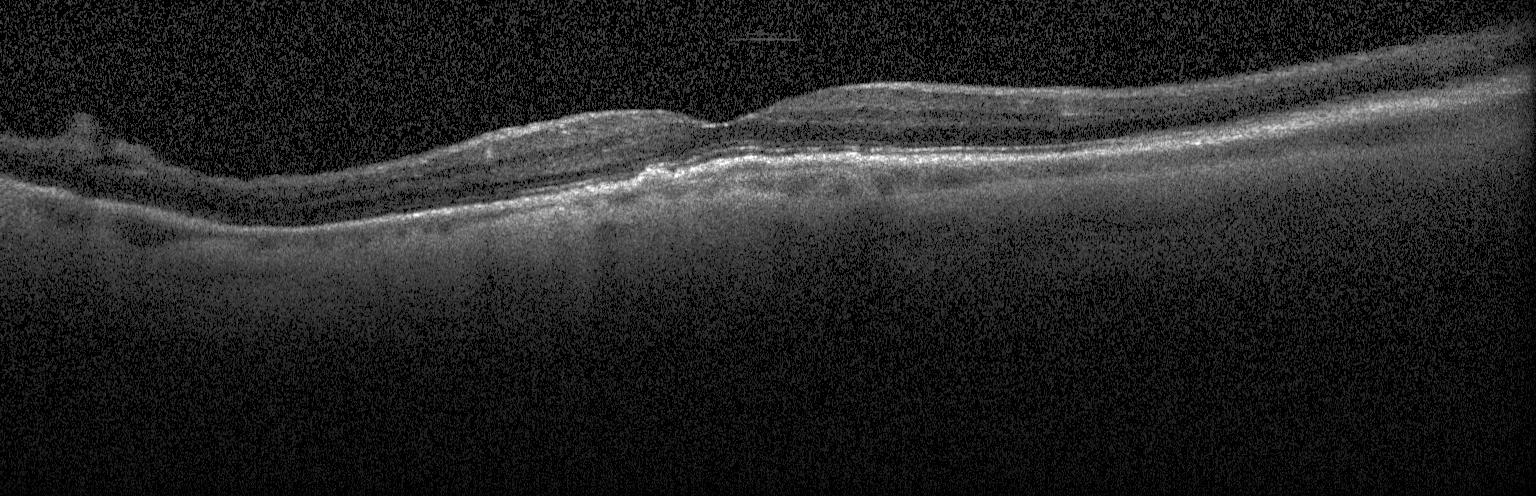 A choroidal neovascular membrane.